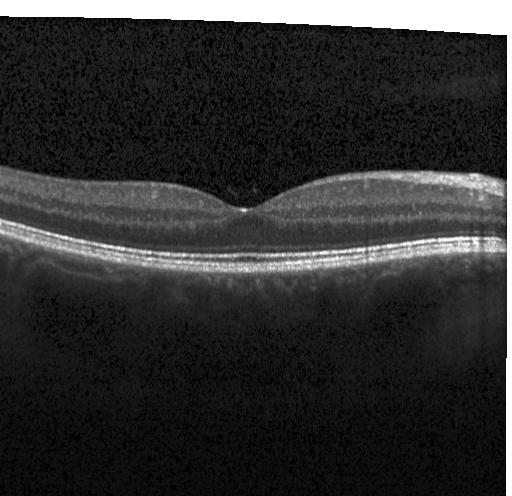 Retinal OCT B-scan. OCT finding: no evidence of choroidal neovascularization, diabetic macular edema, or drusen.